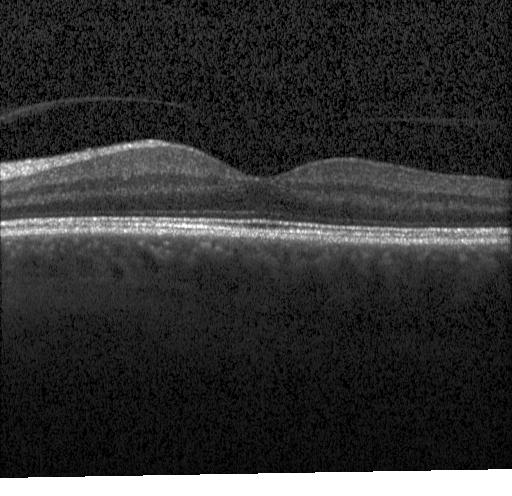
Fovea-centered, OCT line scan. Impression: neither choroidal neovascularization, diabetic macular edema, nor drusen.